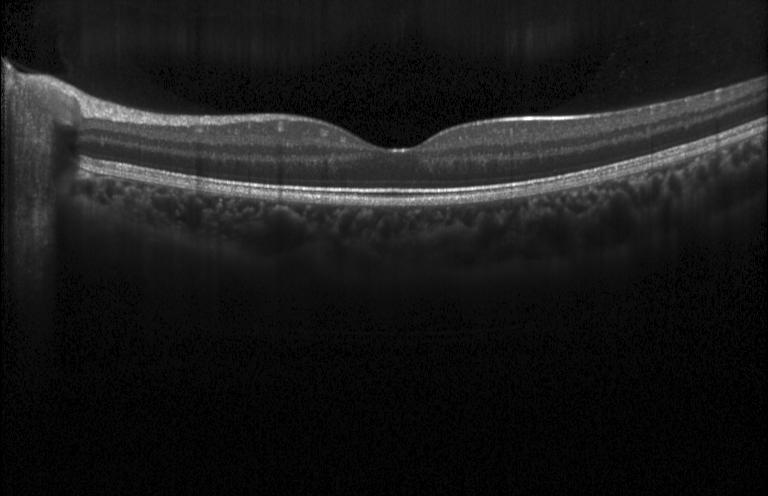
Retinal OCT cross-section, through the macula, Heidelberg Spectralis OCT system.
This B-scan demonstrates neither choroidal neovascularization, diabetic macular edema, nor drusen.